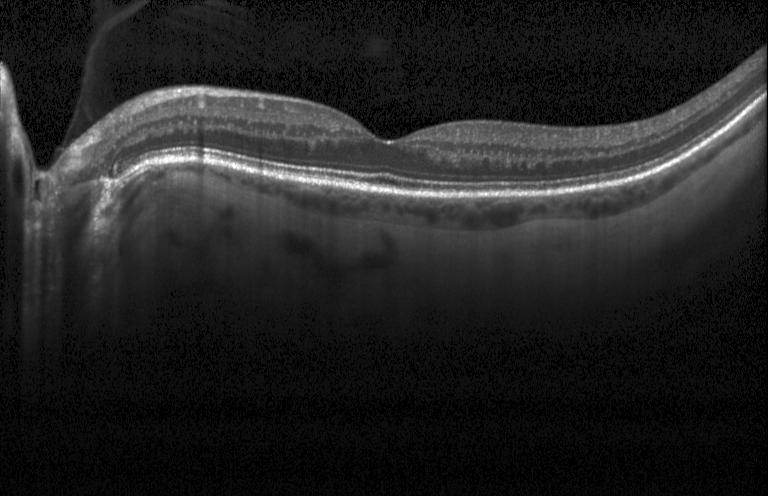

Centered on the fovea; optical coherence tomography B-scan; spectral-domain OCT; Heidelberg Spectralis OCT system
Neither choroidal neovascularization, diabetic macular edema, nor drusen.